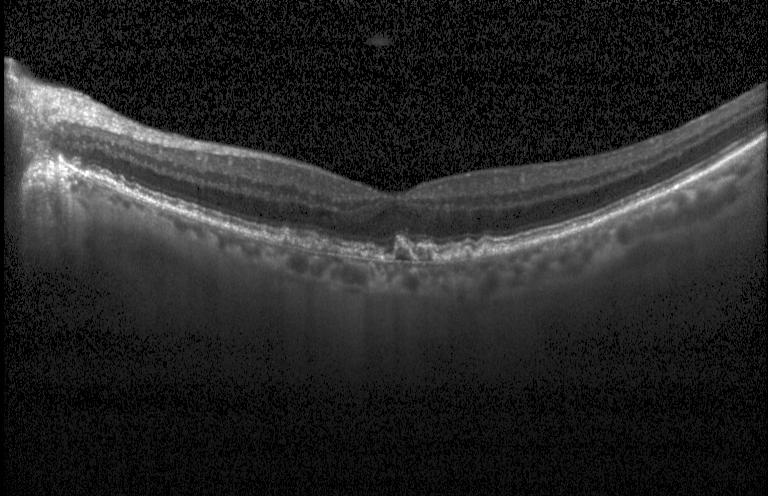

OCT B-scan
This B-scan demonstrates multiple drusen.